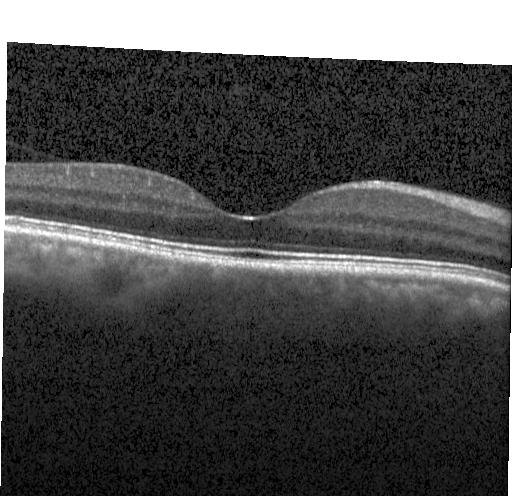 Retinal OCT cross-section · horizontal scan through the fovea.
Finding: no choroidal neovascularization, diabetic macular edema, or drusen.